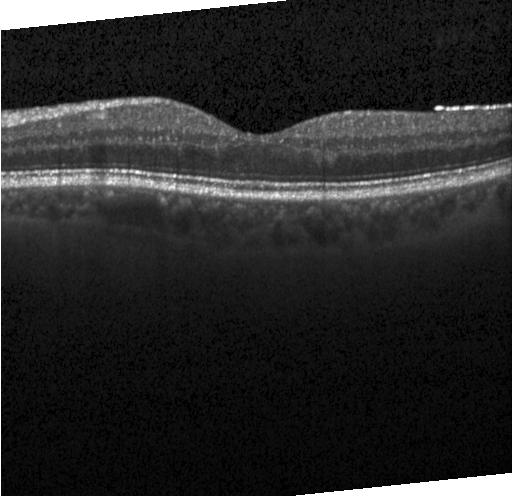

Finding: no CNV, no DME, and no drusen.